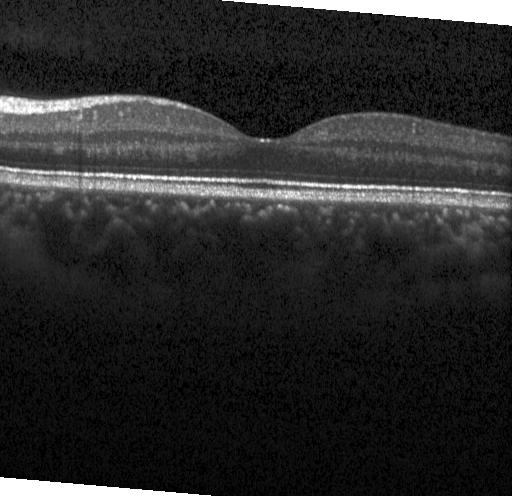
OCT scan showing no evidence of choroidal neovascularization, diabetic macular edema, or drusen.